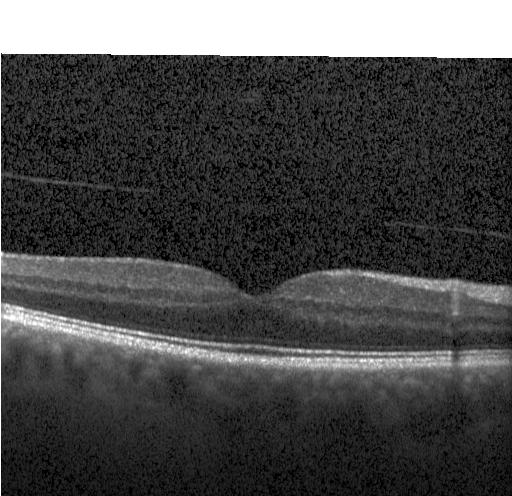

Centered on the fovea, Heidelberg Spectralis, OCT line scan, spectral-domain OCT. Dx: no choroidal neovascularization, diabetic macular edema, or drusen.